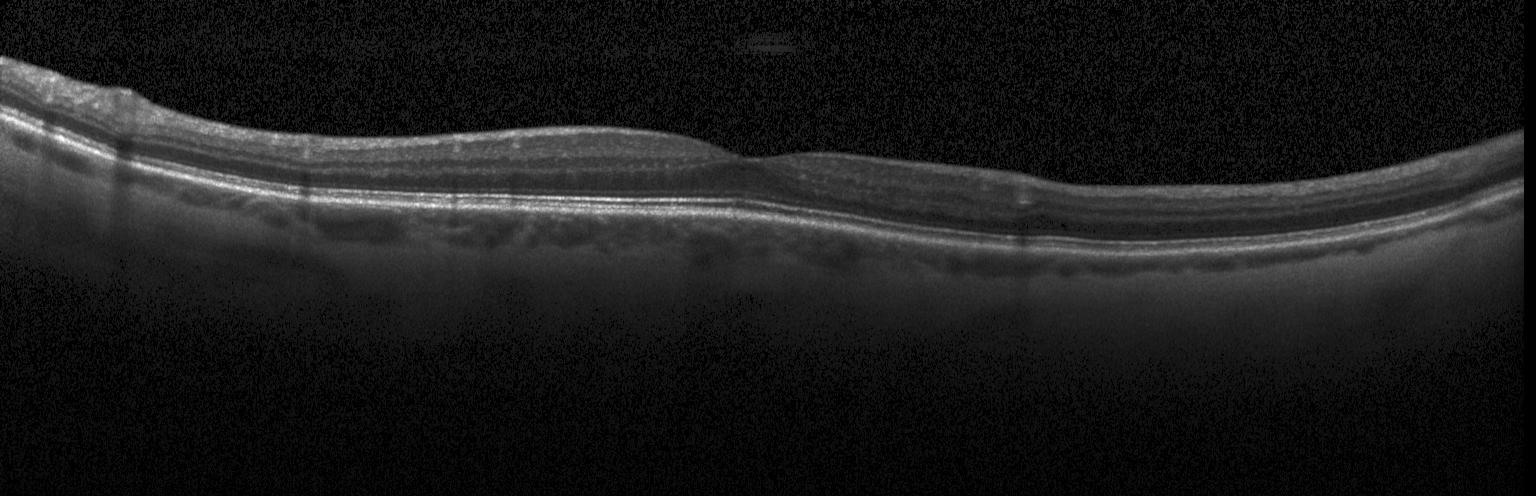 Dx: no evidence of choroidal neovascularization, diabetic macular edema, or drusen.